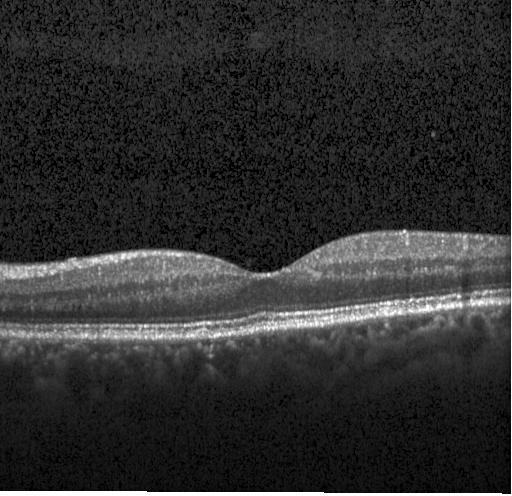 Optical coherence tomography B-scan.
Finding: no choroidal neovascularization, diabetic macular edema, or drusen.